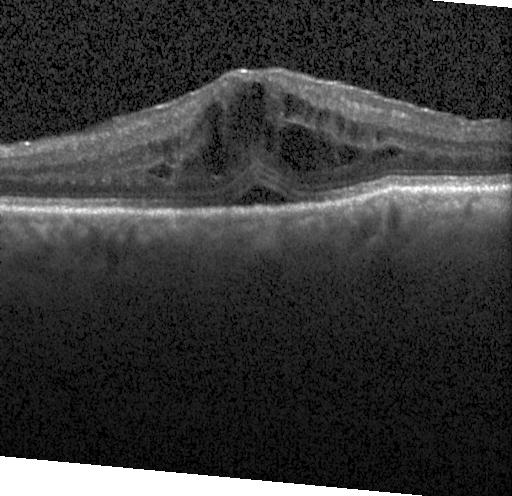 OCT finding: diabetic macular edema.